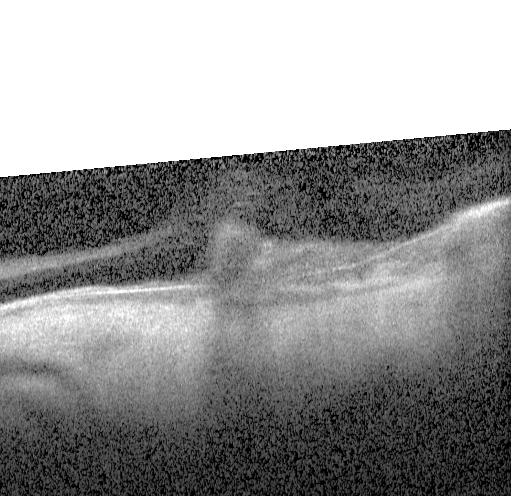

Dx: choroidal neovascularization.